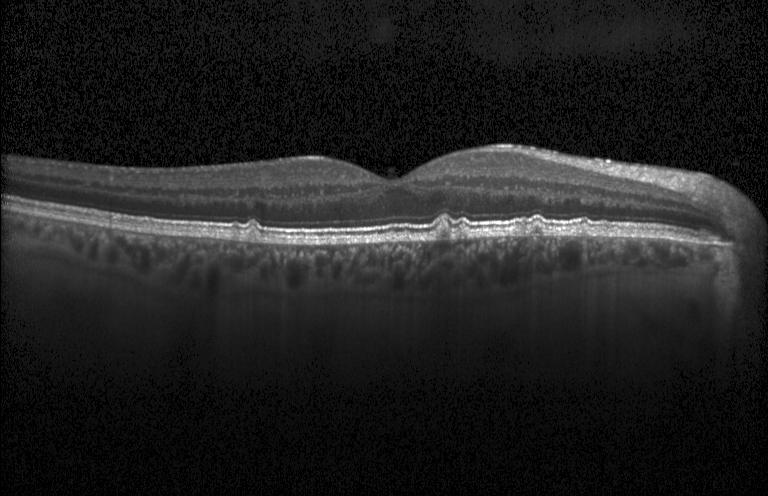

Impression: drusen.